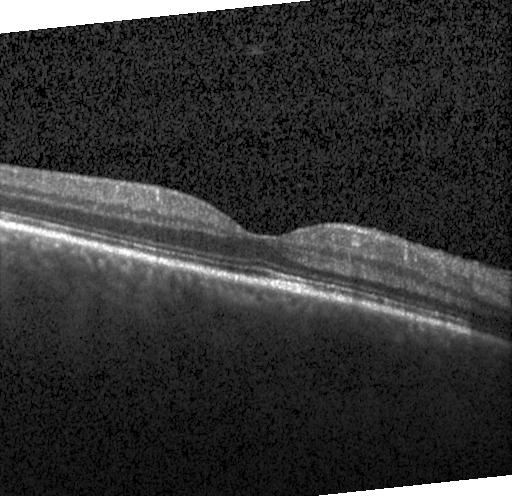
SD-OCT · retinal OCT B-scan · acquired on a Heidelberg Spectralis — Finding: no choroidal neovascularization, no diabetic macular edema, and no drusen.